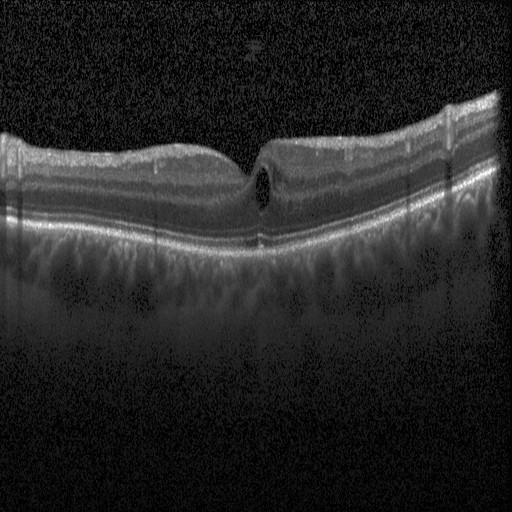

Macular OCT: diabetic macular edema.